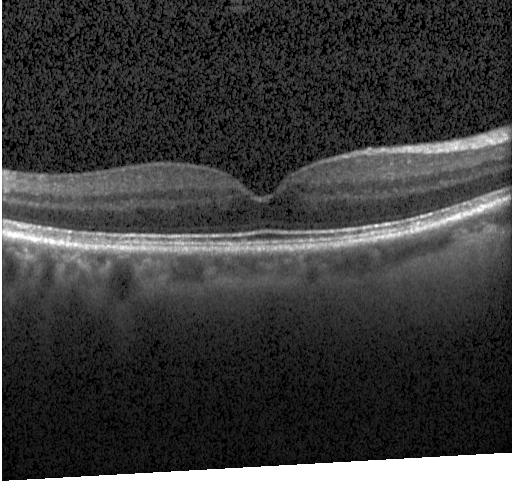
No choroidal neovascularization, no diabetic macular edema, and no drusen.